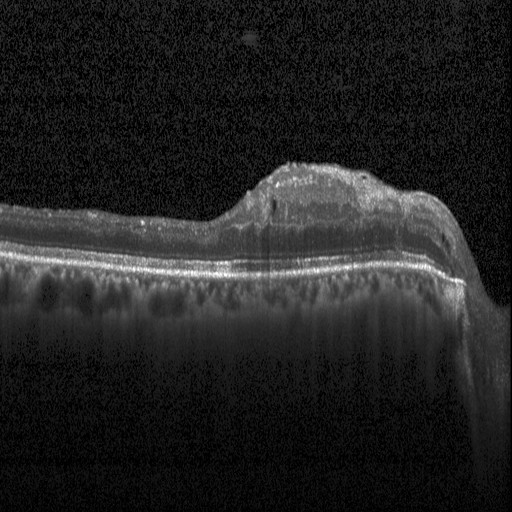

This B-scan demonstrates DME.